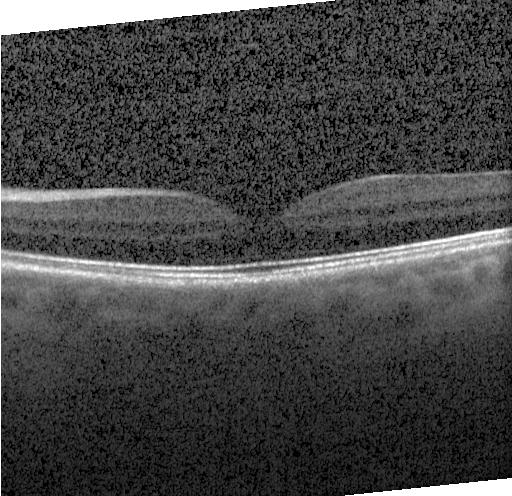

Through the macula. Heidelberg Spectralis. OCT B-scan. Finding: no CNV, DME, or drusen.